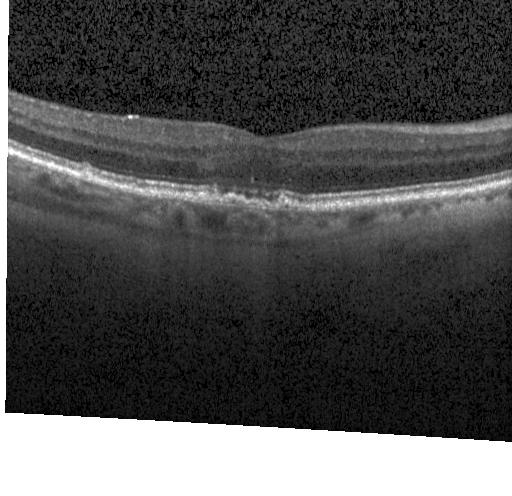
Instrument: Heidelberg Spectralis, macular scan, spectral-domain optical coherence tomography, OCT line scan.
Diagnosis: multiple drusen.